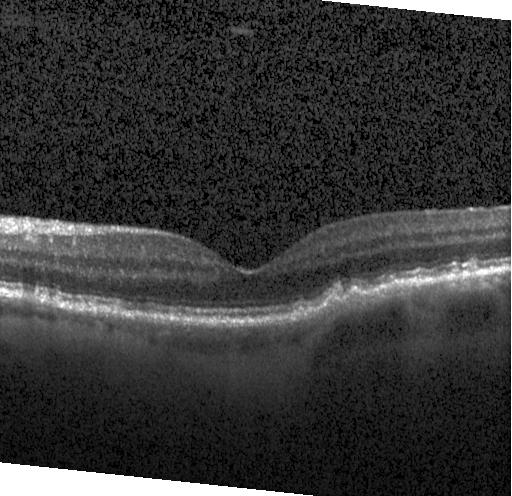 Dx: sub-RPE drusenoid deposits.